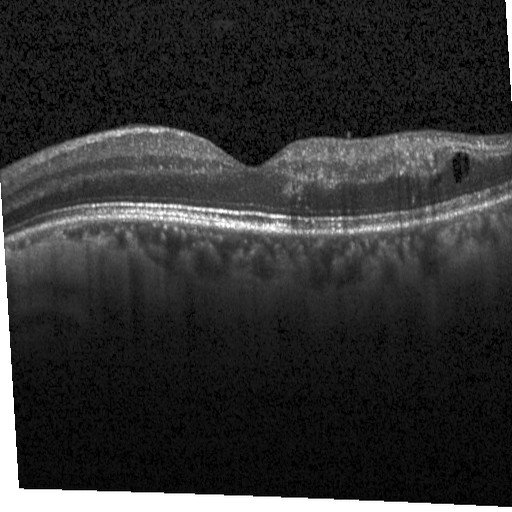

Horizontal scan through the fovea. Retinal OCT cross-section. Spectral-domain OCT. Acquired on a Heidelberg Spectralis
Dx: DME.